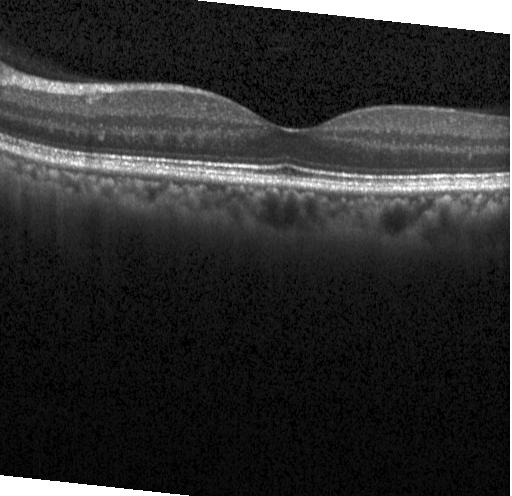

Retinal OCT B-scan. Impression: no CNV, no DME, and no drusen.